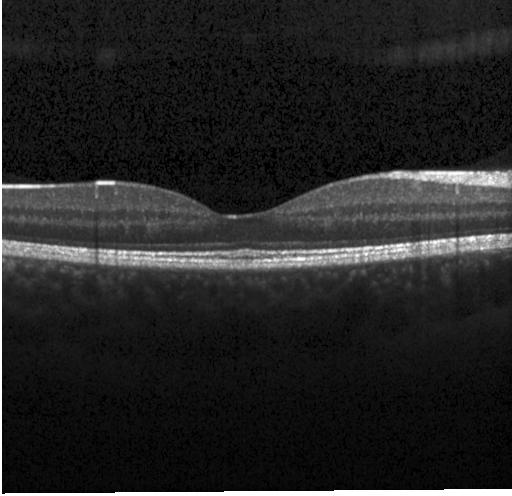 OCT line scan, SD-OCT.
Assessment: neither CNV, DME, nor drusen.